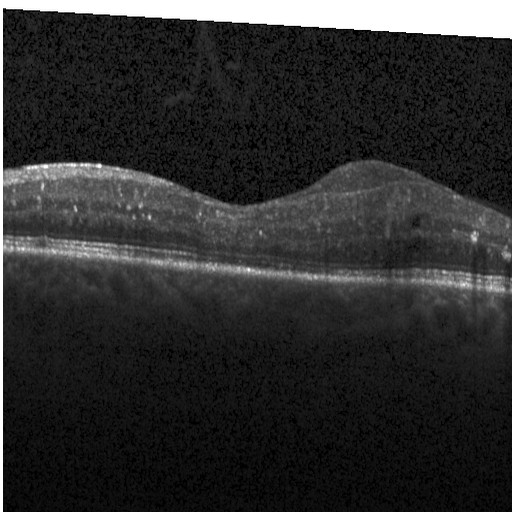
Acquired on a Heidelberg Spectralis, OCT line scan, spectral-domain optical coherence tomography. Finding: diabetic macular edema (DME).